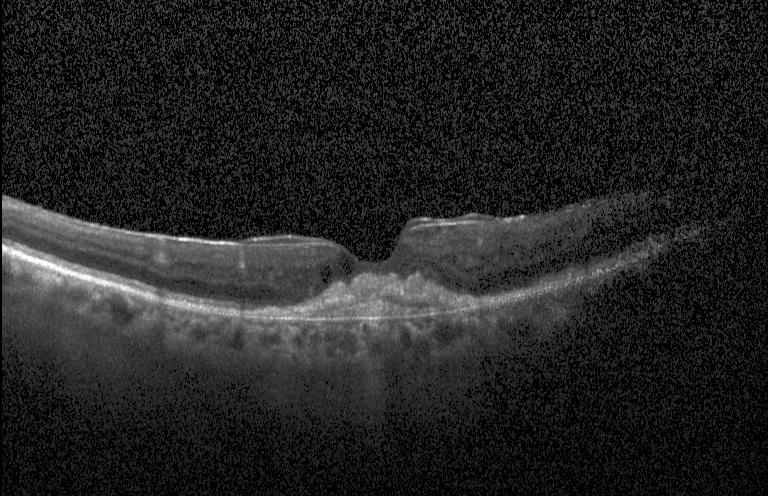

Heidelberg Spectralis; SD-OCT; optical coherence tomography B-scan; fovea-centered. OCT finding: choroidal neovascularization.